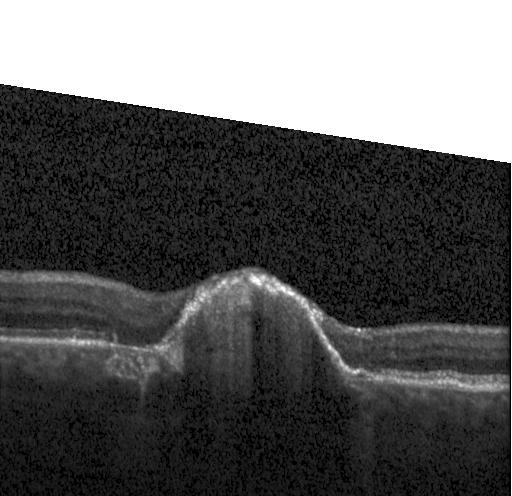 OCT line scan, spectral-domain optical coherence tomography. This B-scan demonstrates a choroidal neovascular membrane.